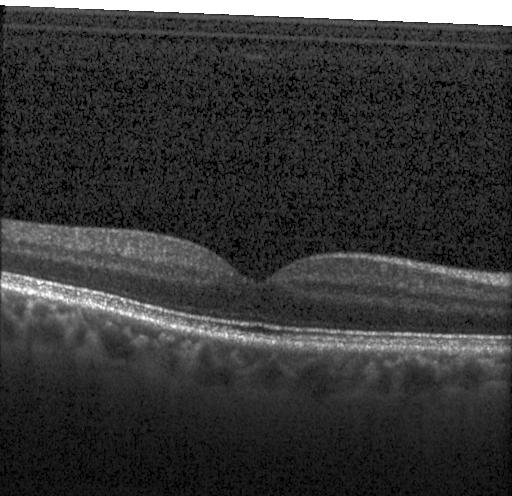
OCT finding: no evidence of choroidal neovascularization, diabetic macular edema, or drusen.